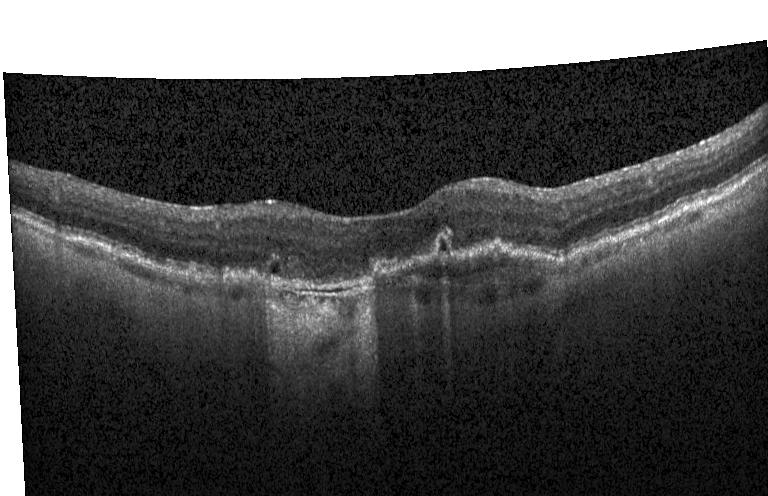 Diagnosis: a choroidal neovascular membrane.